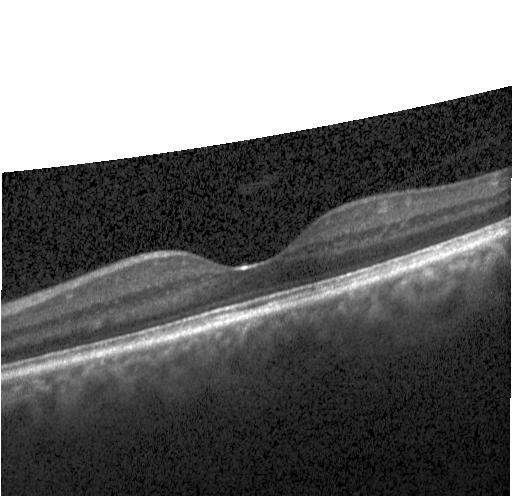 OCT finding: neither CNV, DME, nor drusen.